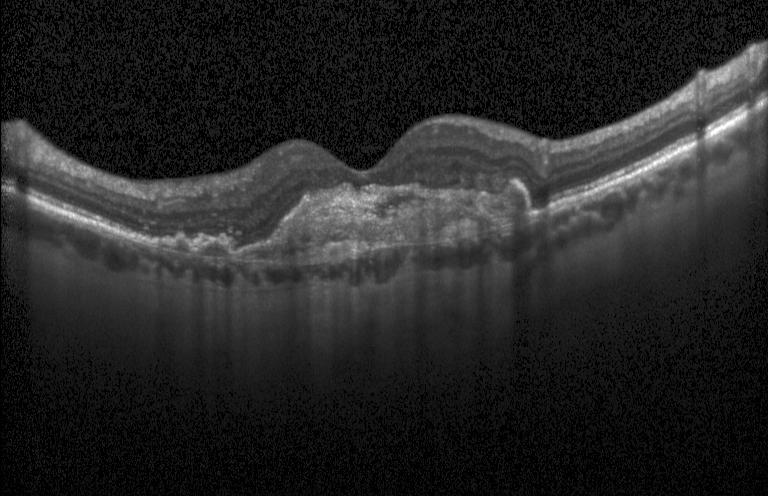

Diagnosis: a choroidal neovascular membrane.